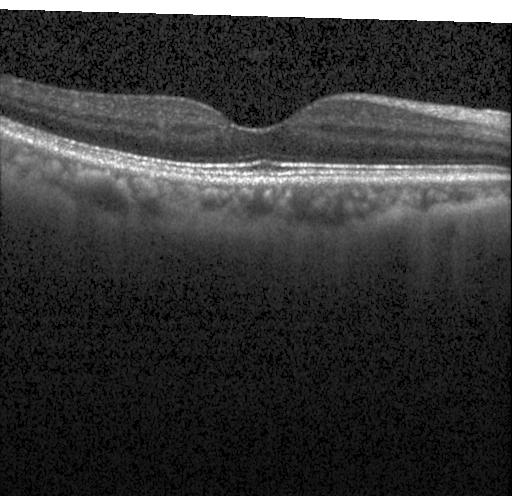

Centered on the fovea, optical coherence tomography scan, acquired on a Heidelberg Spectralis, spectral-domain OCT. This B-scan demonstrates no choroidal neovascularization, diabetic macular edema, or drusen.